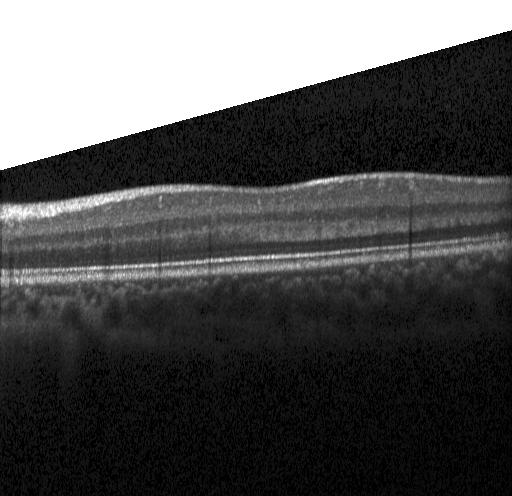 Retinal OCT B-scan. Dx: no evidence of CNV, DME, or drusen.